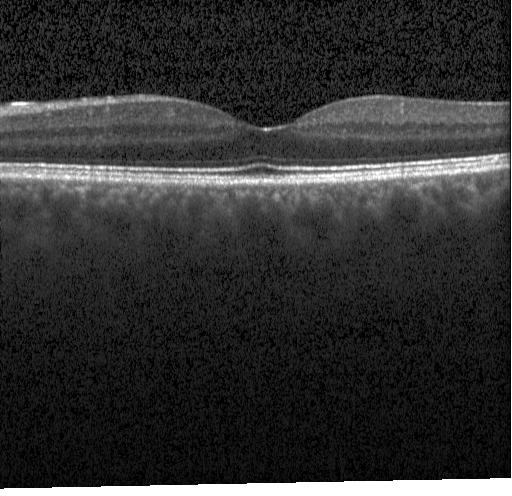

SD-OCT, optical coherence tomography B-scan.
Impression: neither choroidal neovascularization, diabetic macular edema, nor drusen.